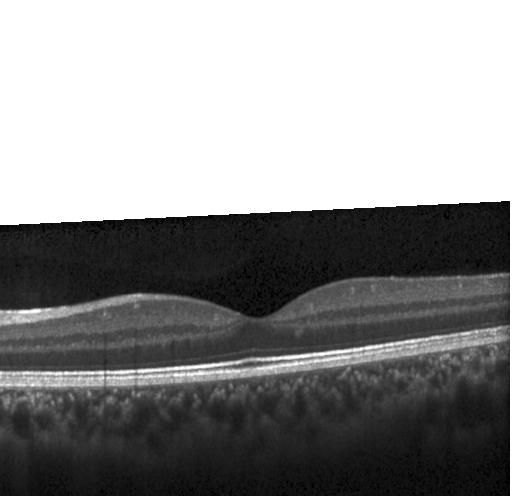 Impression: no evidence of CNV, DME, or drusen.